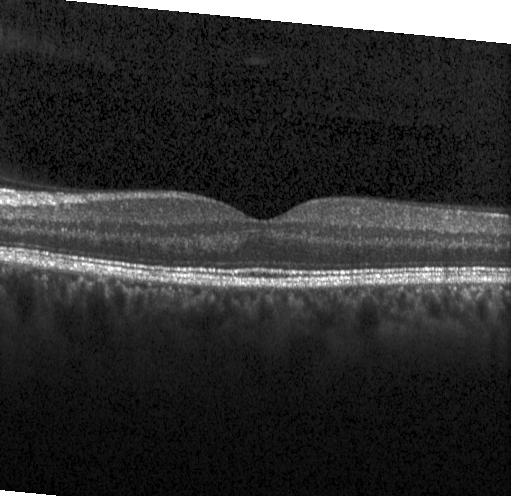

OCT line scan; Heidelberg Spectralis; macular scan — Impression: neither choroidal neovascularization, diabetic macular edema, nor drusen.